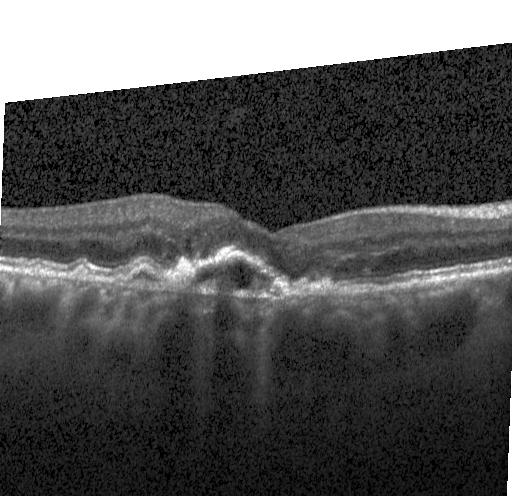 Fovea-centered, optical coherence tomography scan, spectral-domain OCT
Diagnosis: choroidal neovascularization (CNV).